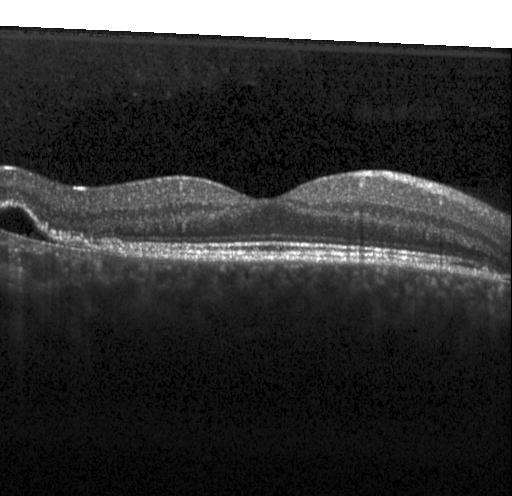 Retinal OCT B-scan. Impression: a choroidal neovascular membrane.